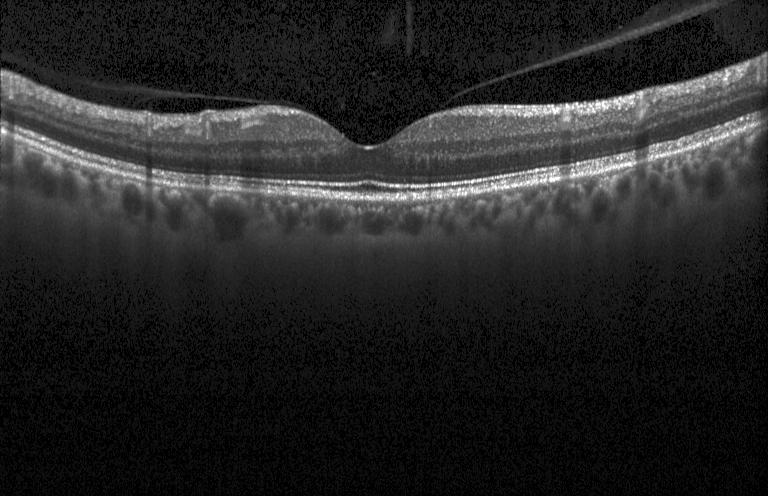
Retinal OCT B-scan. Dx: no choroidal neovascularization, no diabetic macular edema, and no drusen.